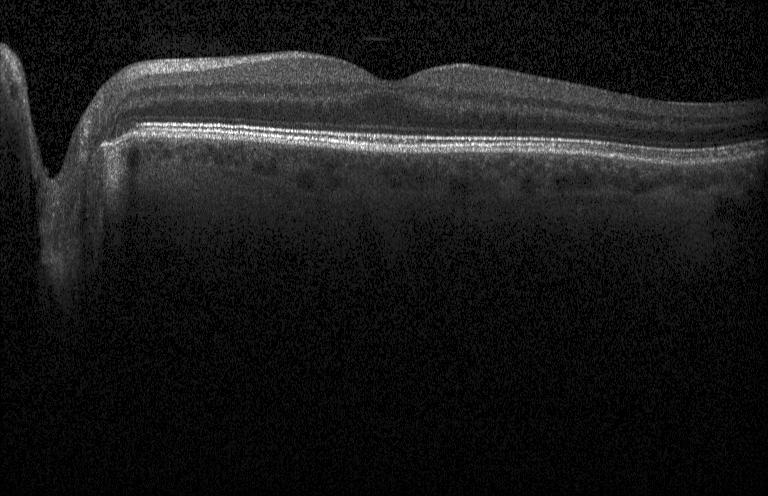

Instrument: Heidelberg Spectralis. Through the macula. Retinal OCT cross-section. Spectral-domain OCT.
Assessment: neither CNV, DME, nor drusen.